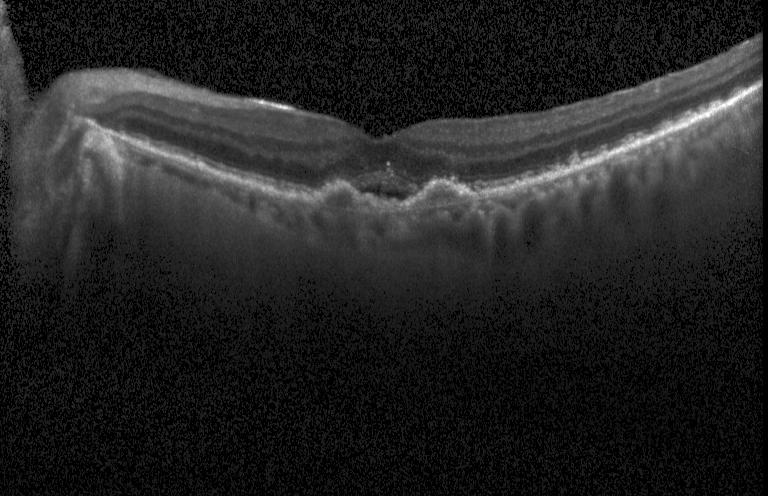 Spectral-domain optical coherence tomography; Heidelberg Spectralis; retinal OCT cross-section; through the macula. The scan shows choroidal neovascularization.